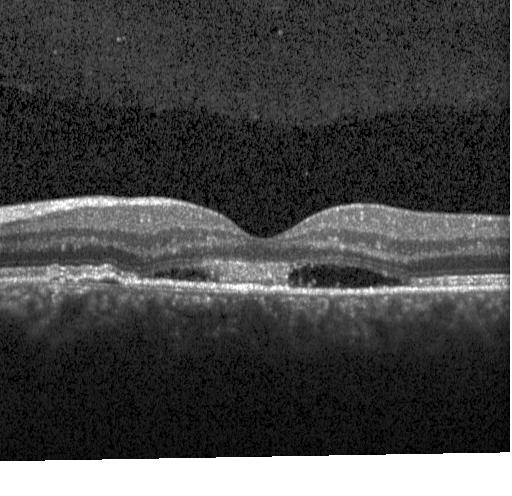

Through the macula. OCT B-scan — The scan shows a choroidal neovascular membrane.